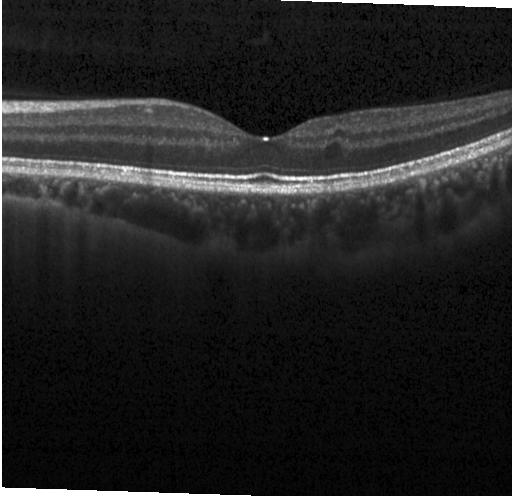
Optical coherence tomography scan
The scan shows no choroidal neovascularization, diabetic macular edema, or drusen.